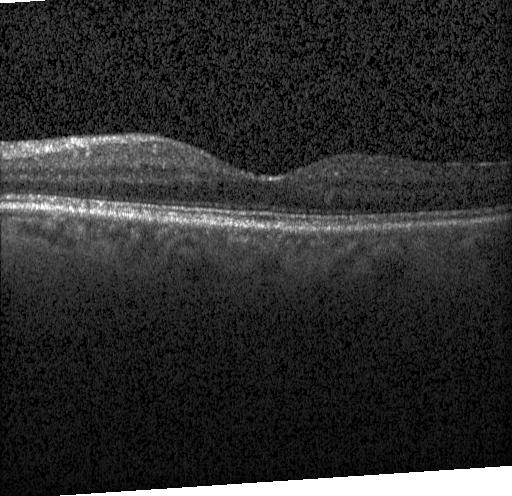

Macular scan · optical coherence tomography scan. This B-scan demonstrates no CNV, DME, or drusen.